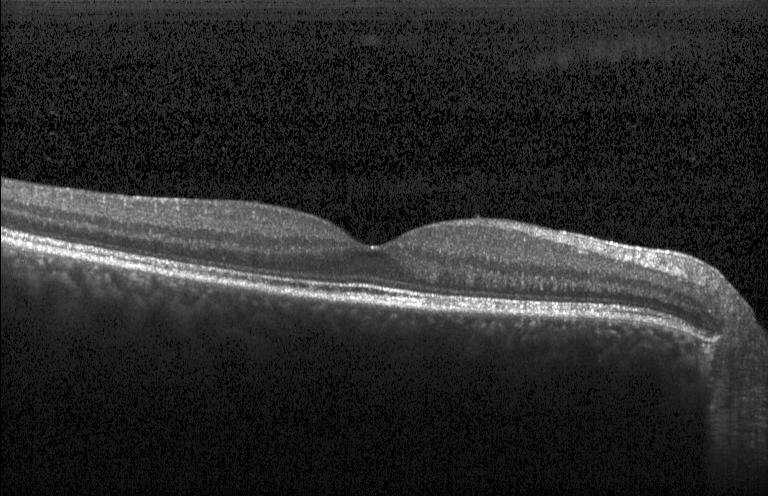

Centered on the fovea. Spectral-domain OCT. Heidelberg Spectralis. Optical coherence tomography scan — Impression: no CNV, DME, or drusen.